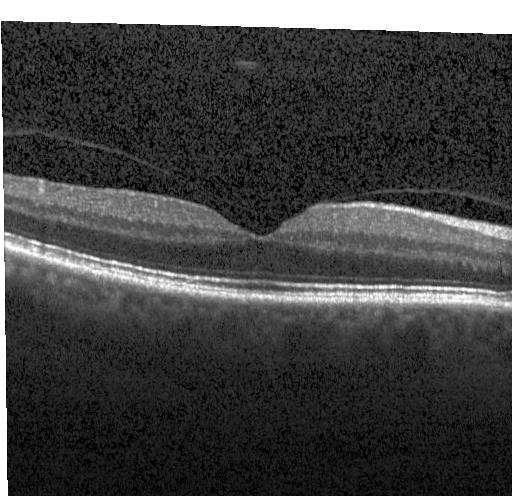
Spectral-domain OCT B-scan: neither choroidal neovascularization, diabetic macular edema, nor drusen.